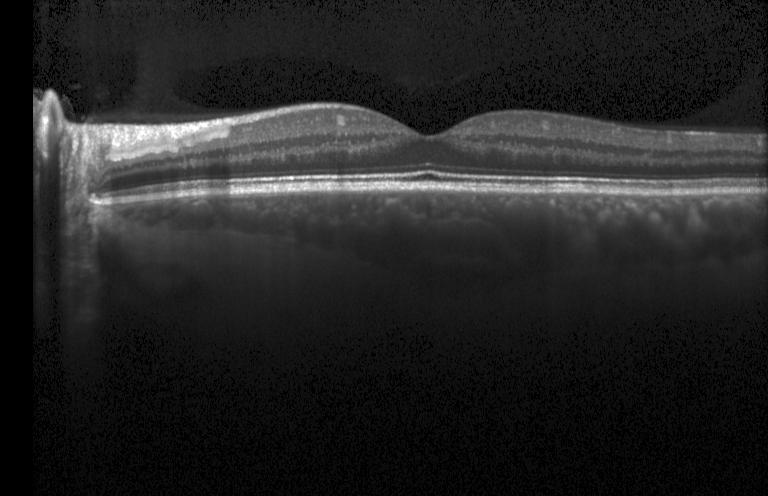
No CNV, DME, or drusen.